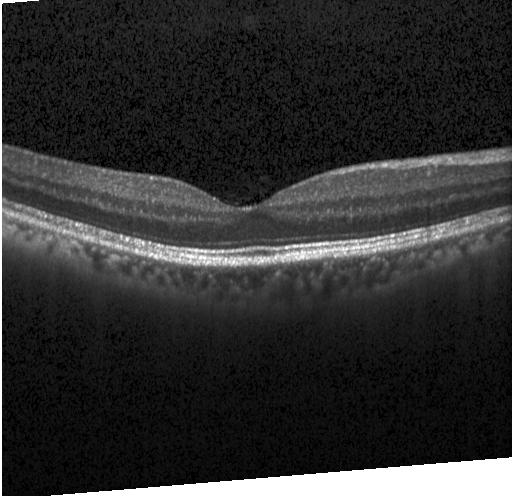

OCT finding: neither choroidal neovascularization, diabetic macular edema, nor drusen.